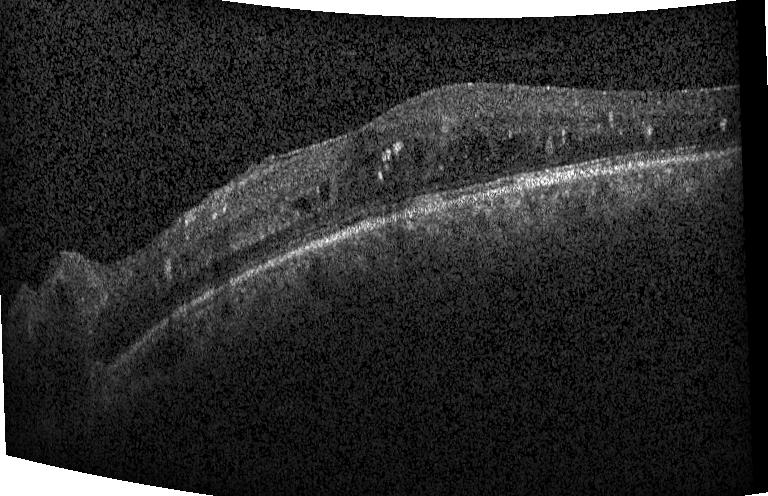 Dx: DME.